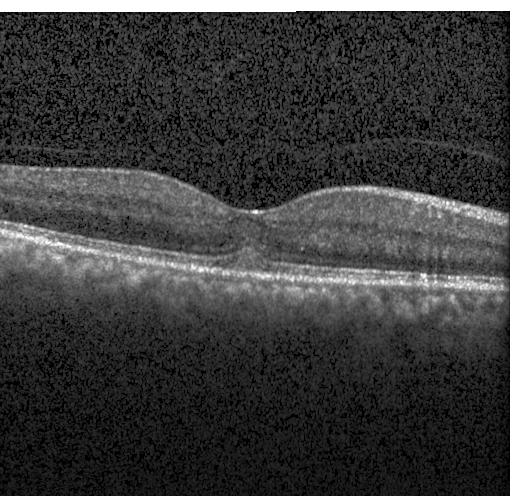
Optical coherence tomography scan; spectral-domain OCT. Assessment: a choroidal neovascular membrane.